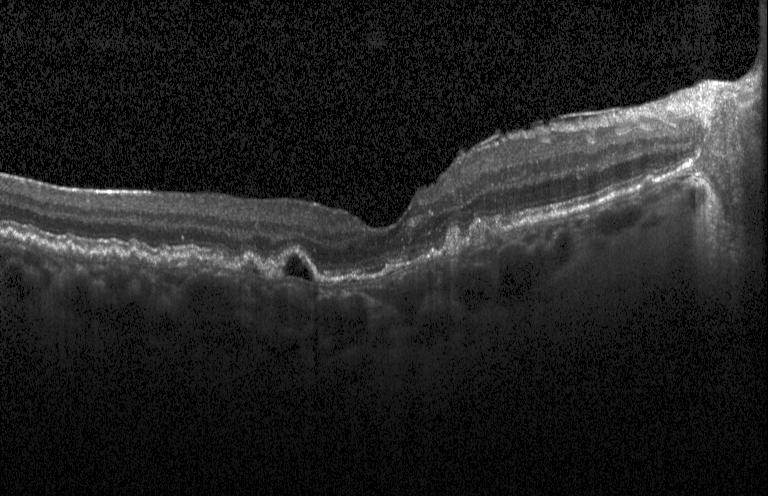
OCT B-scan showing a choroidal neovascular membrane.